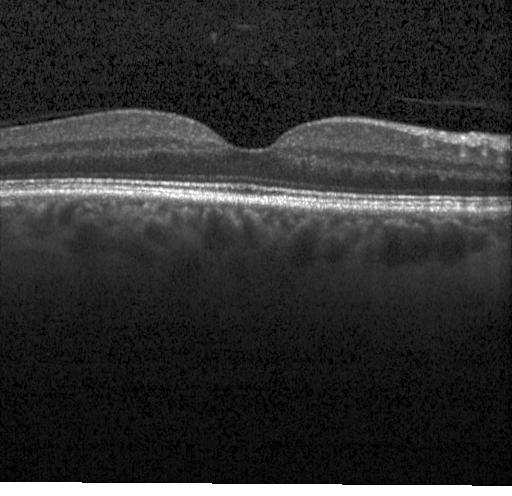 Through the macula, acquired on a Heidelberg Spectralis, SD-OCT, retinal OCT cross-section.
Dx: no CNV, DME, or drusen.